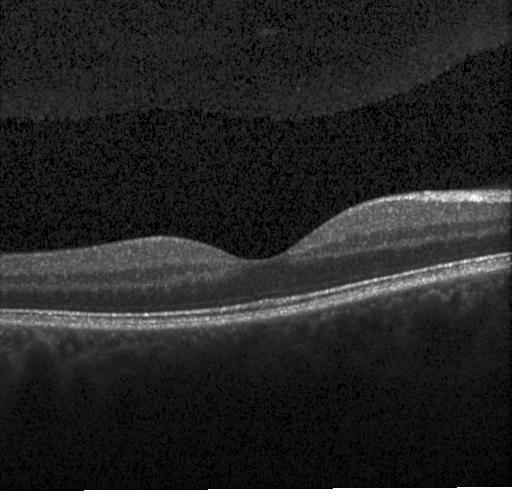

Diagnosis: no evidence of CNV, DME, or drusen.